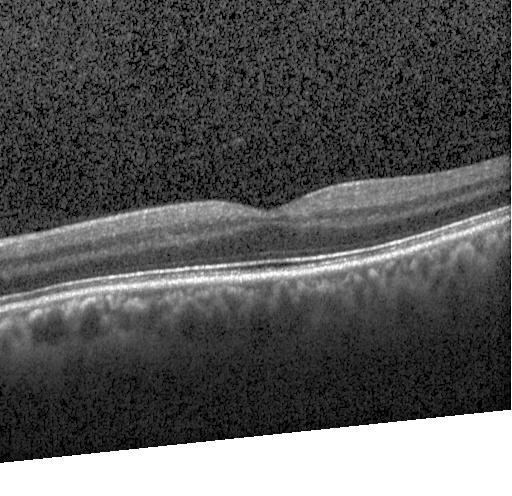
Acquired on a Heidelberg Spectralis, optical coherence tomography B-scan, spectral-domain OCT, horizontal scan through the fovea — The scan shows no choroidal neovascularization, diabetic macular edema, or drusen.